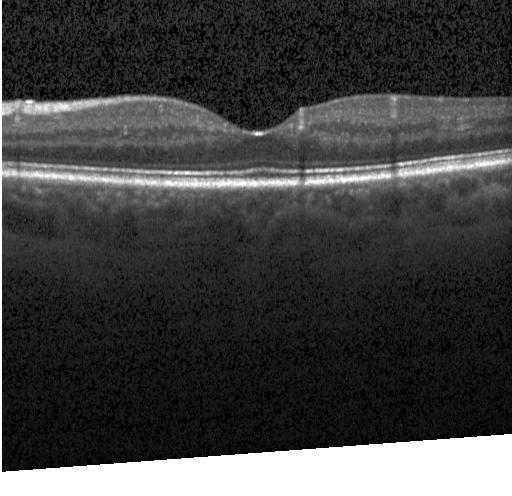

Instrument: Heidelberg Spectralis · spectral-domain optical coherence tomography · optical coherence tomography B-scan — Impression: neither choroidal neovascularization, diabetic macular edema, nor drusen.